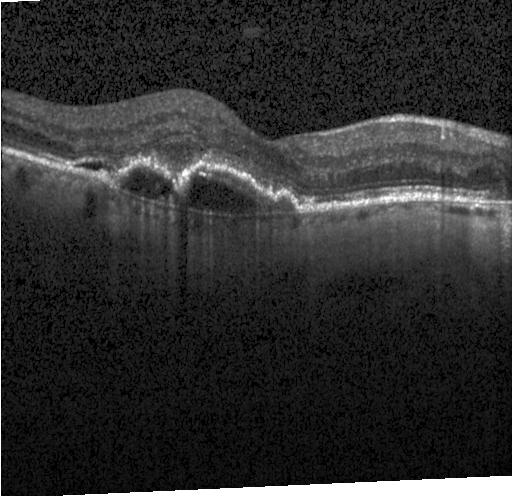

SD-OCT. Retinal OCT B-scan — Diagnosis: choroidal neovascularization.